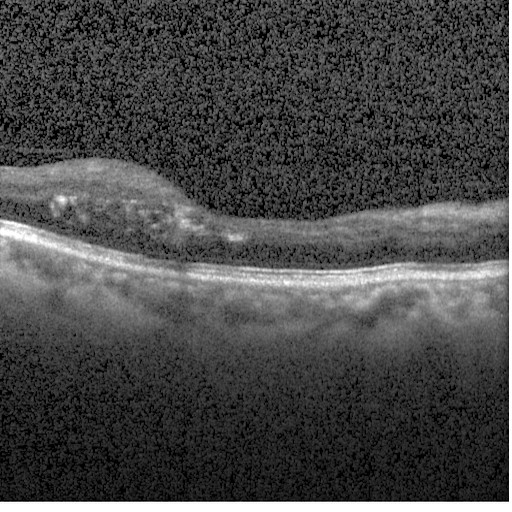 OCT finding: diabetic macular edema (DME).